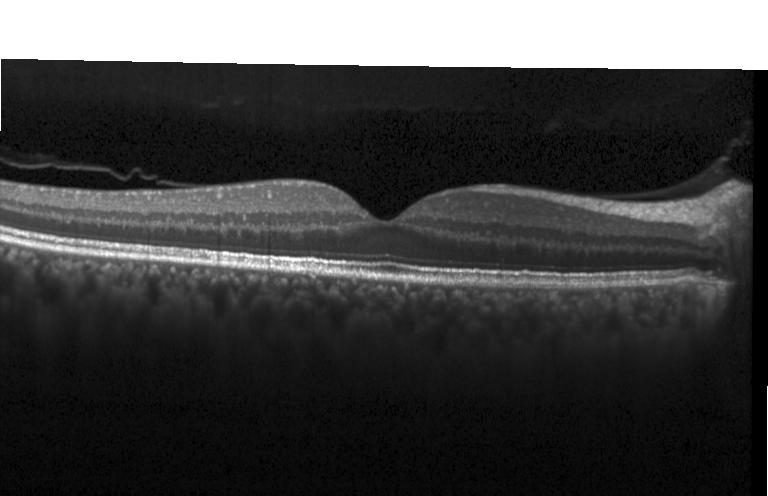

Spectral-domain OCT B-scan: no evidence of choroidal neovascularization, diabetic macular edema, or drusen.